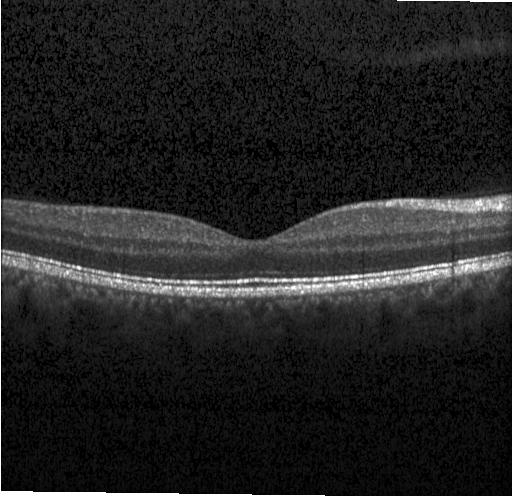 Impression: no CNV, DME, or drusen.